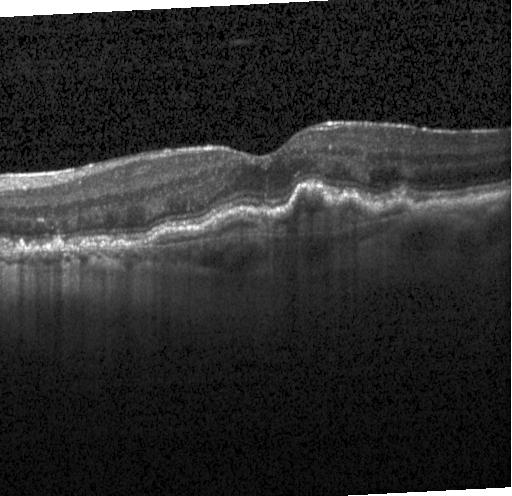 OCT B-scan. Choroidal neovascularization (CNV).